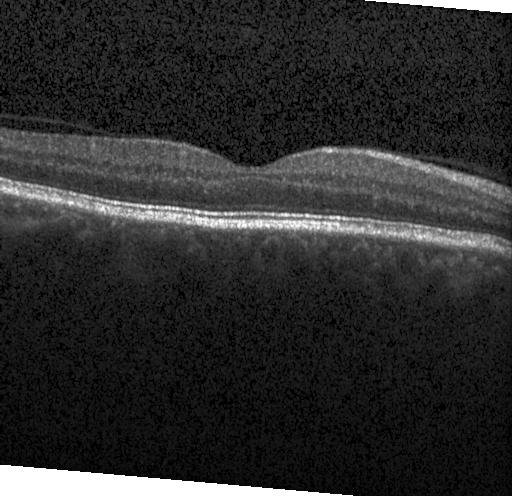
OCT finding: neither CNV, DME, nor drusen.